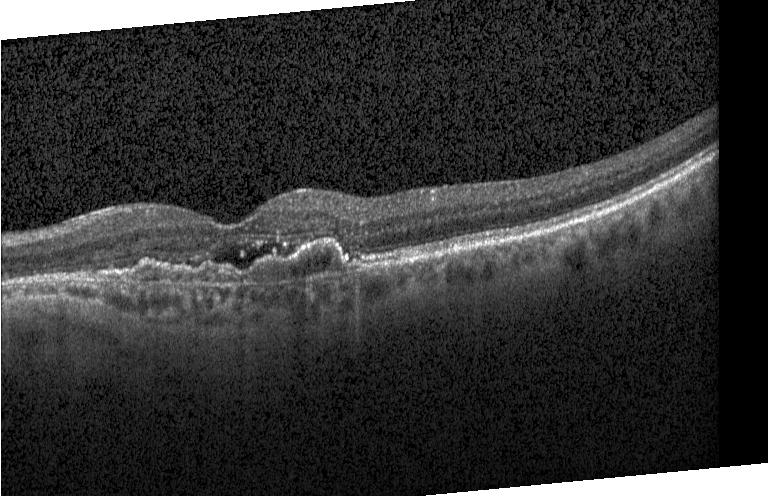
Optical coherence tomography B-scan
Assessment: choroidal neovascularization.